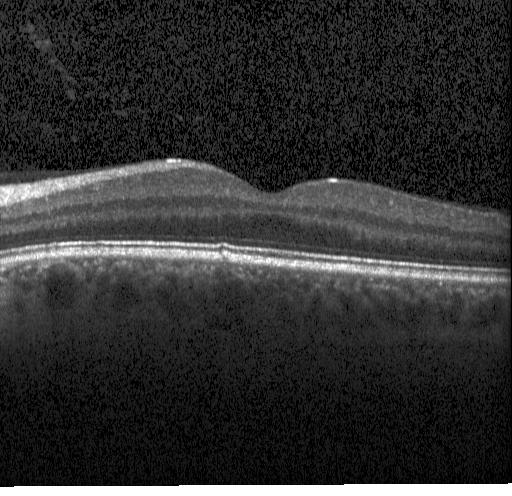

Dx: sub-RPE drusenoid deposits.